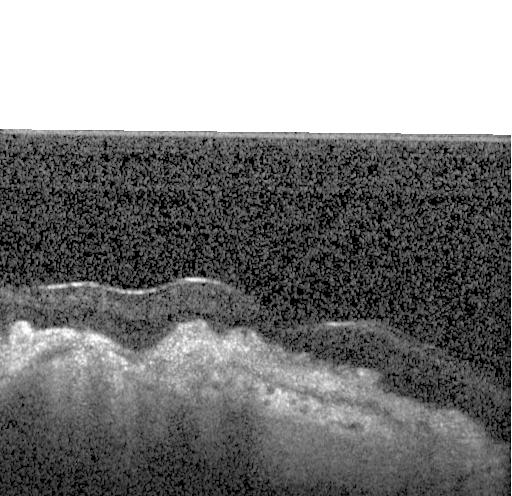

Macular OCT: choroidal neovascularization (CNV).